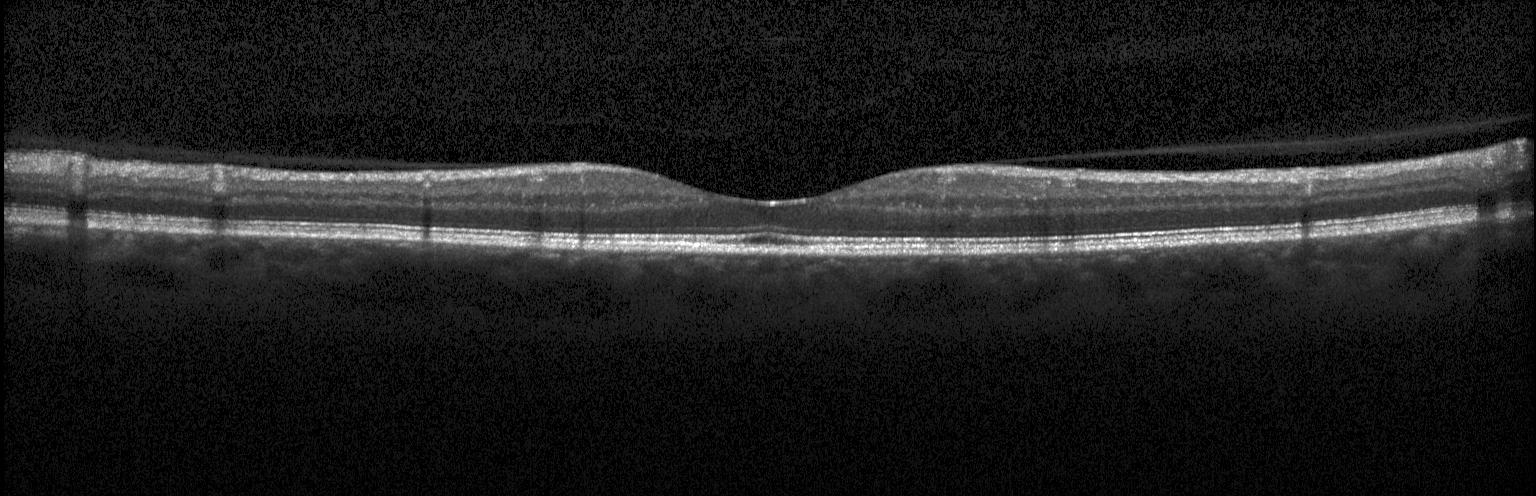 Retinal OCT cross-section. Macular OCT: neither choroidal neovascularization, diabetic macular edema, nor drusen.